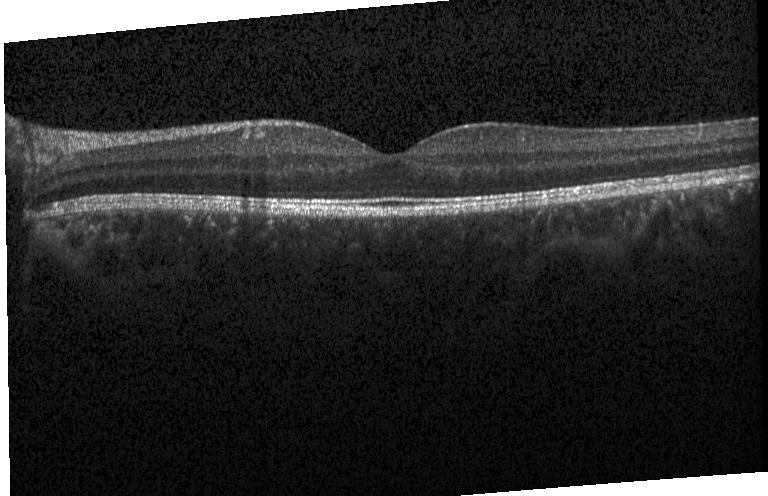
Acquired on a Heidelberg Spectralis, retinal OCT B-scan, fovea-centered — Finding: neither CNV, DME, nor drusen.